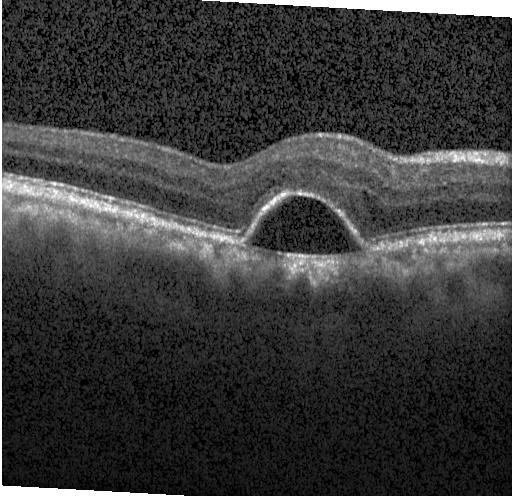

SD-OCT · through the macula · retinal OCT B-scan · Heidelberg Spectralis OCT system. The scan shows choroidal neovascularization (CNV).